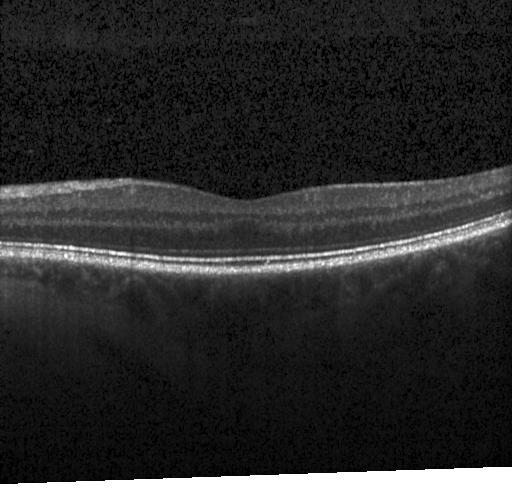
OCT B-scan; Heidelberg Spectralis; spectral-domain OCT; horizontal scan through the fovea. This B-scan demonstrates neither choroidal neovascularization, diabetic macular edema, nor drusen.